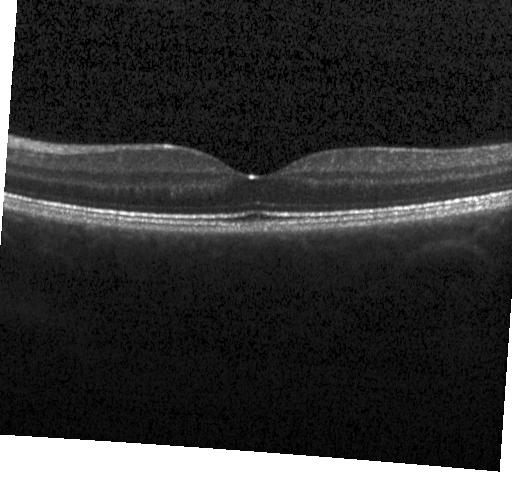
Retinal OCT B-scan; spectral-domain OCT. Impression: neither CNV, DME, nor drusen.